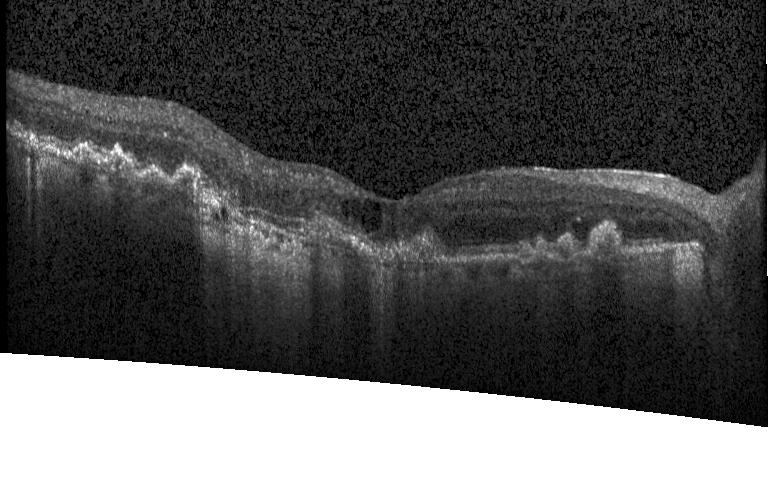

Retinal OCT cross-section, spectral-domain optical coherence tomography. Diagnosis: choroidal neovascularization.